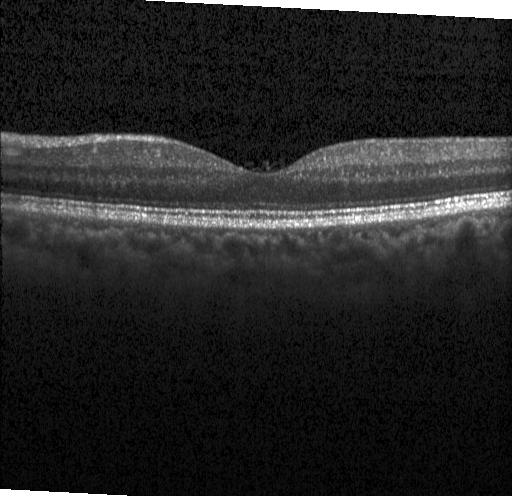

Fovea-centered · Heidelberg Spectralis · optical coherence tomography B-scan. The scan shows no evidence of CNV, DME, or drusen.